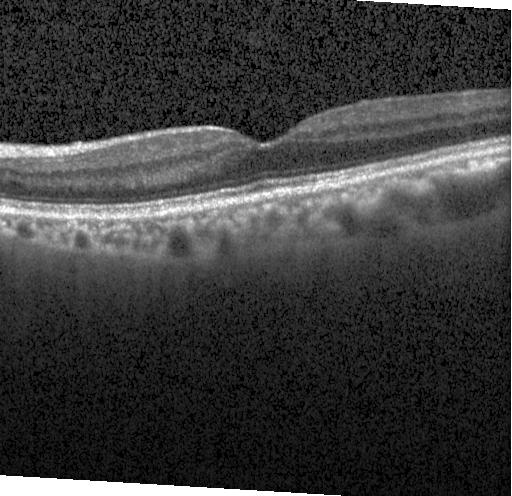

Heidelberg Spectralis; optical coherence tomography scan — OCT finding: no choroidal neovascularization, diabetic macular edema, or drusen.